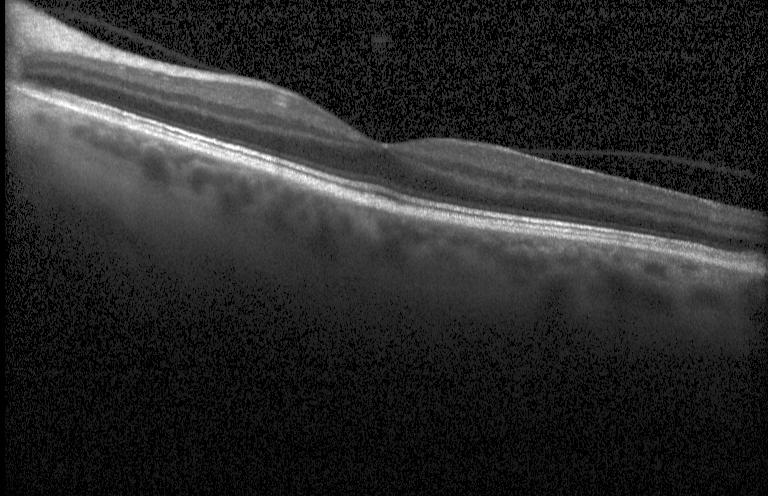
The scan shows neither choroidal neovascularization, diabetic macular edema, nor drusen.